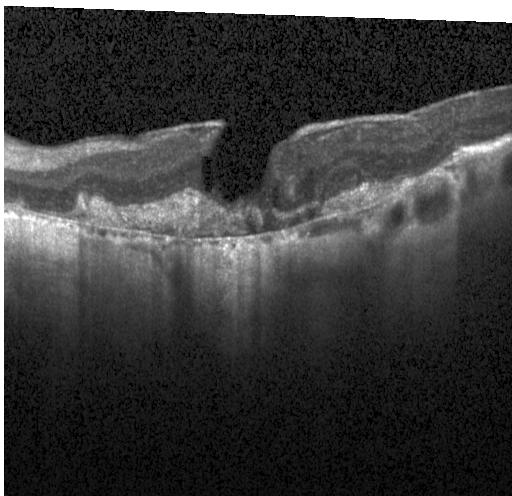 Retinal OCT B-scan
Choroidal neovascularization.